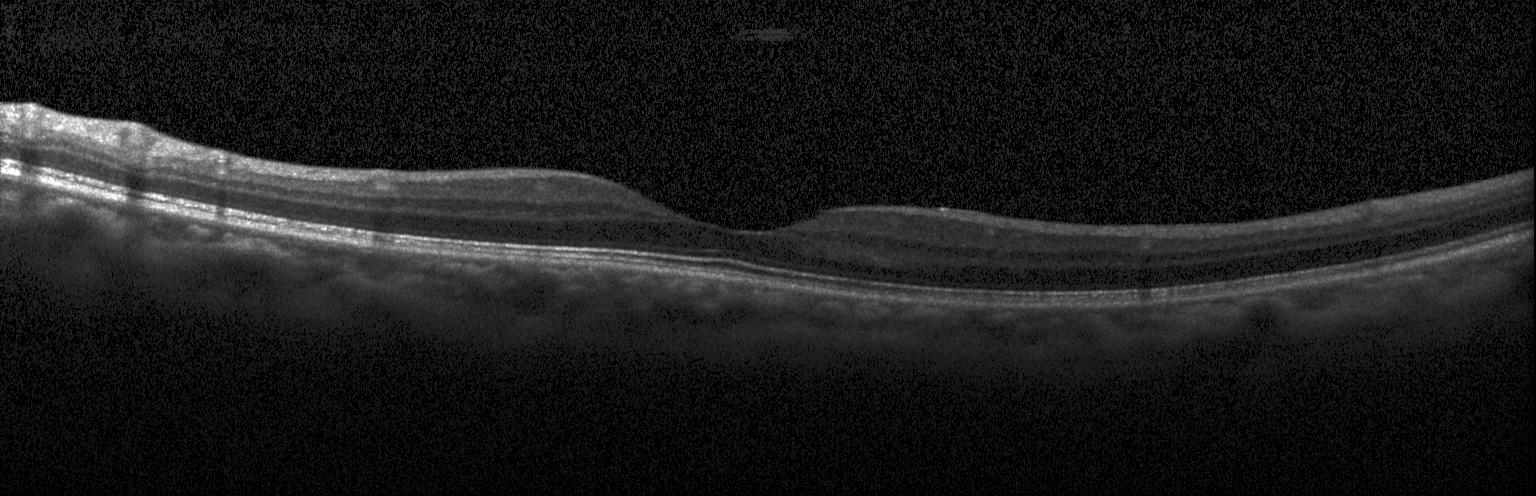

Optical coherence tomography B-scan. This B-scan demonstrates neither CNV, DME, nor drusen.